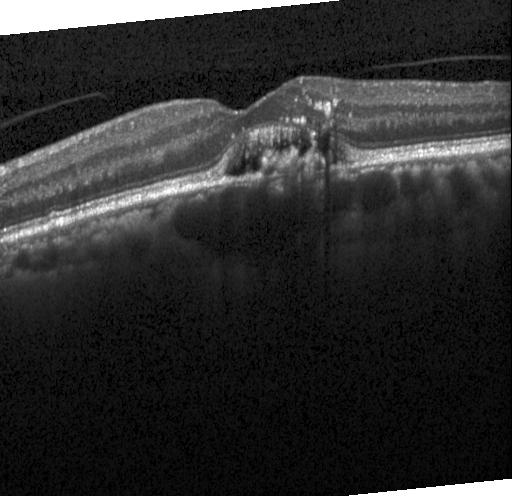

OCT finding: choroidal neovascularization.